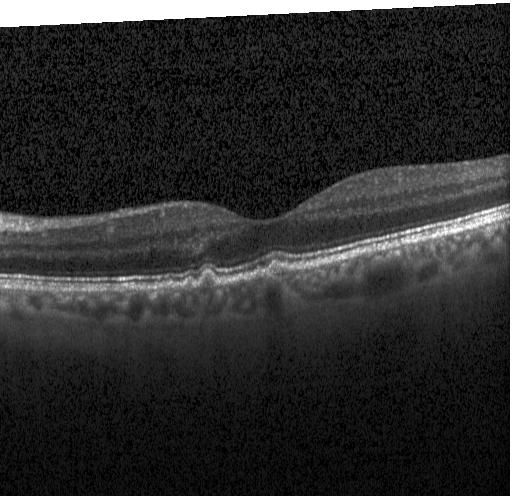 Heidelberg Spectralis · spectral-domain OCT · retinal OCT B-scan
The scan shows sub-RPE drusenoid deposits.